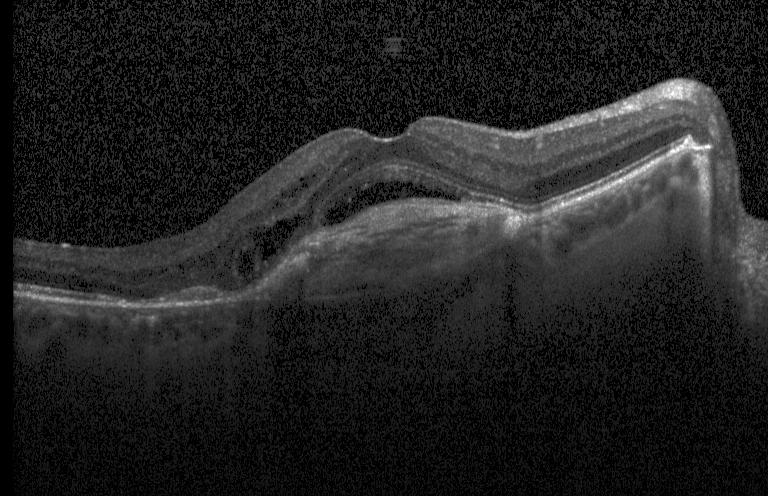
Dx: a choroidal neovascular membrane.